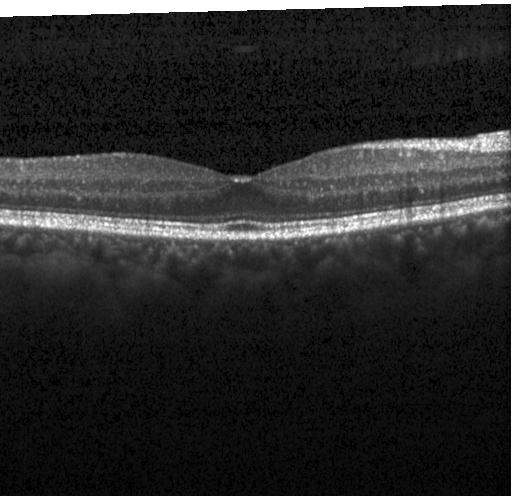

Instrument: Heidelberg Spectralis. Retinal OCT B-scan. Macular scan. Spectral-domain OCT — The scan shows no CNV, no DME, and no drusen.